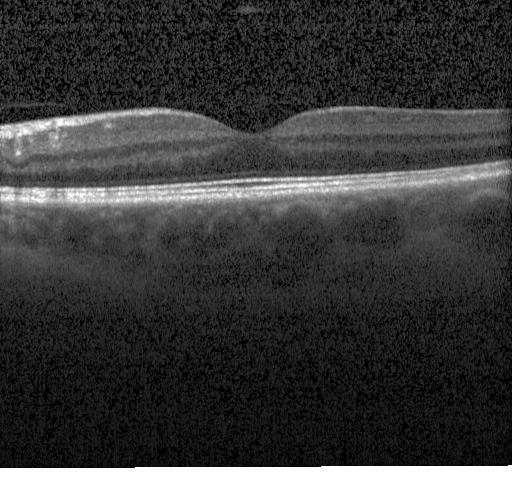

Retinal OCT cross-section, SD-OCT, instrument: Heidelberg Spectralis. Assessment: neither choroidal neovascularization, diabetic macular edema, nor drusen.